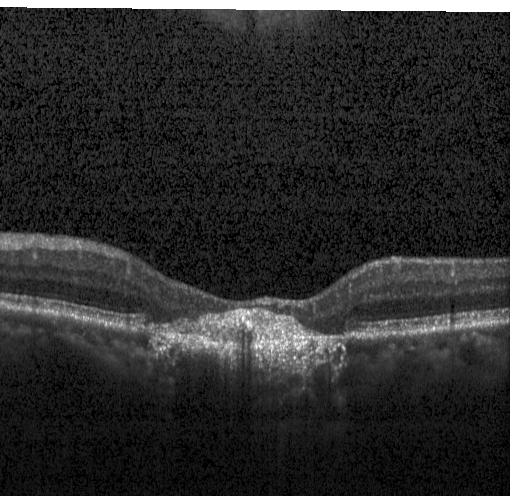 Macular OCT demonstrating CNV.